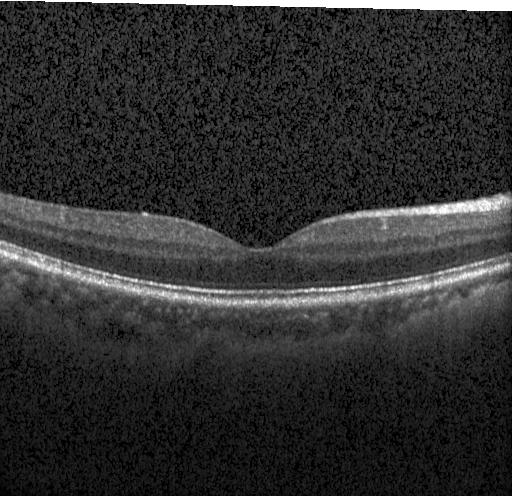
Optical coherence tomography B-scan. No choroidal neovascularization, diabetic macular edema, or drusen.